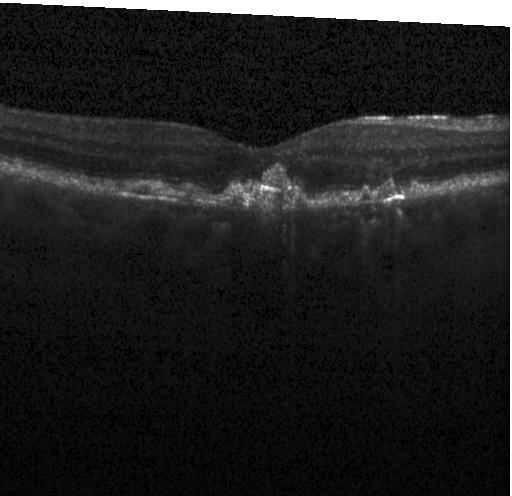

Centered on the fovea, spectral-domain optical coherence tomography, optical coherence tomography scan. This B-scan demonstrates a choroidal neovascular membrane.